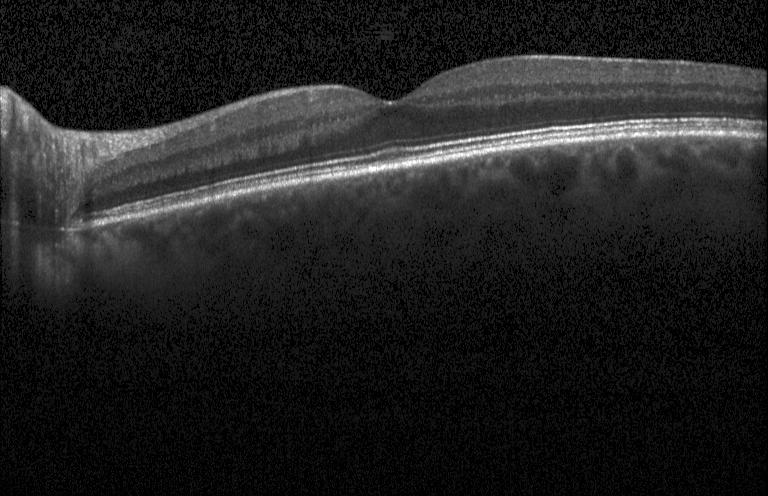 Optical coherence tomography B-scan. Fovea-centered.
No choroidal neovascularization, diabetic macular edema, or drusen.